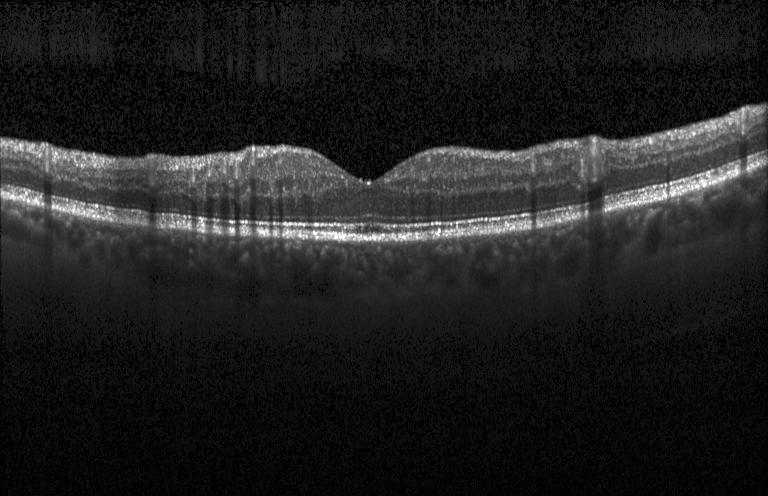
Macular OCT: no choroidal neovascularization, diabetic macular edema, or drusen.